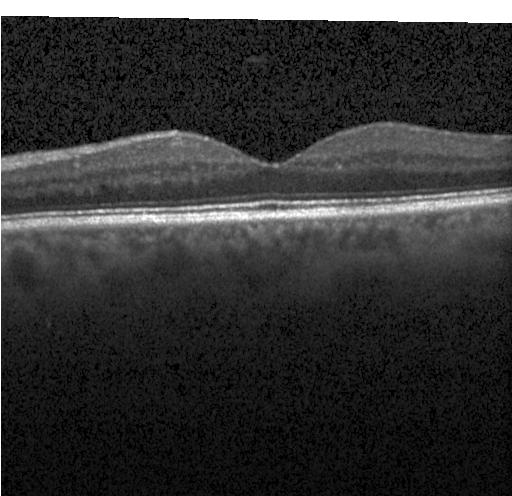 OCT B-scan; instrument: Heidelberg Spectralis.
No choroidal neovascularization, diabetic macular edema, or drusen.